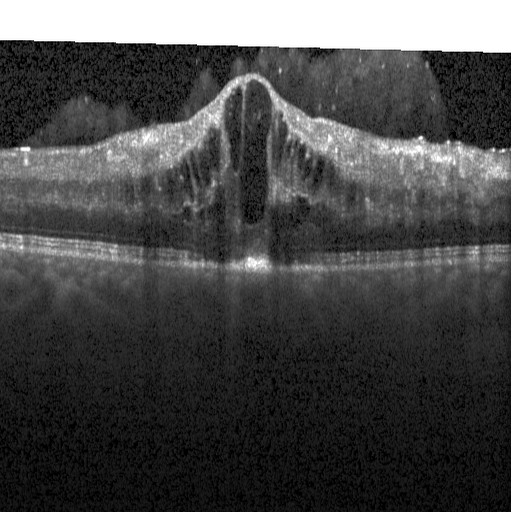
Spectral-domain OCT · OCT line scan. Impression: DME.